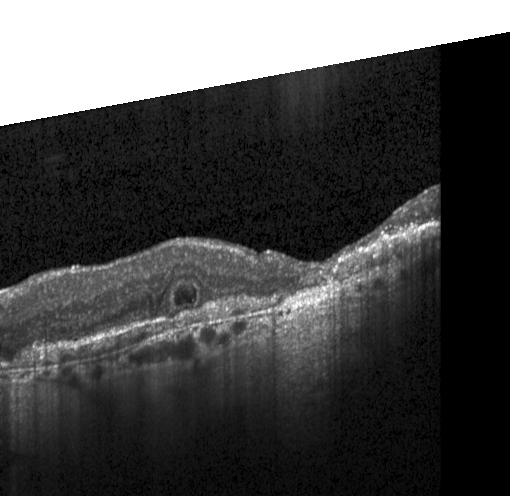

Acquired on a Heidelberg Spectralis, optical coherence tomography scan. Finding: a choroidal neovascular membrane.